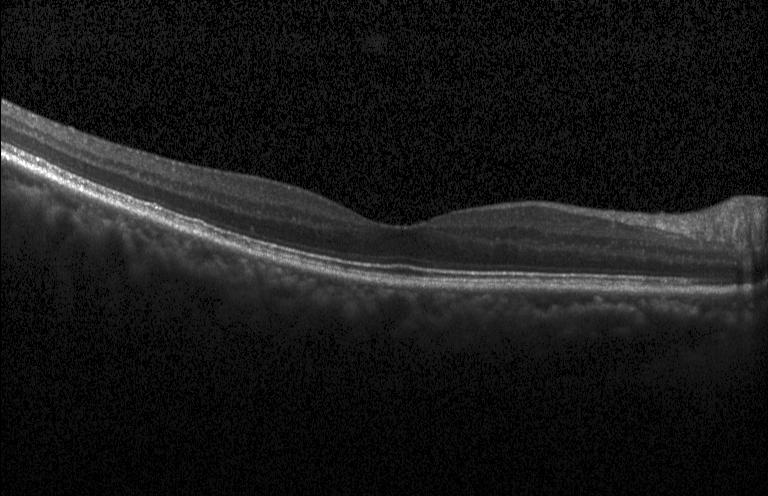 Centered on the fovea · optical coherence tomography B-scan · SD-OCT · Heidelberg Spectralis OCT system. Impression: no CNV, DME, or drusen.